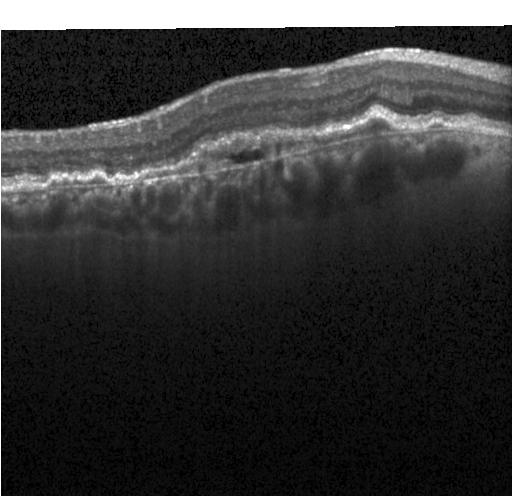 Impression: choroidal neovascularization.